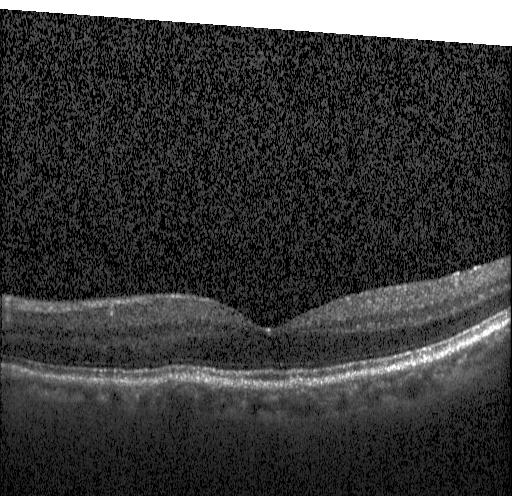
Optical coherence tomography scan.
OCT finding: no evidence of choroidal neovascularization, diabetic macular edema, or drusen.